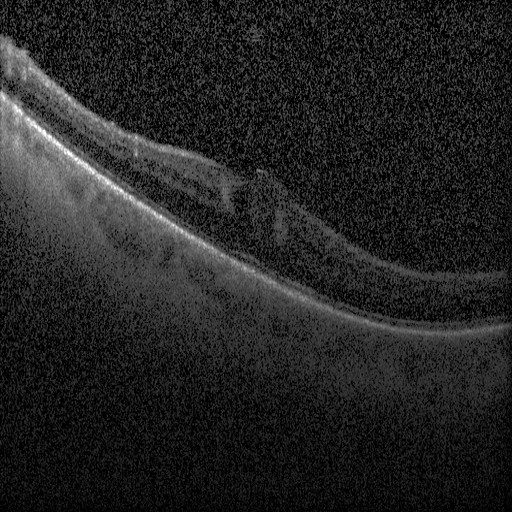

Optical coherence tomography B-scan — Diagnosis: diabetic macular edema (DME).